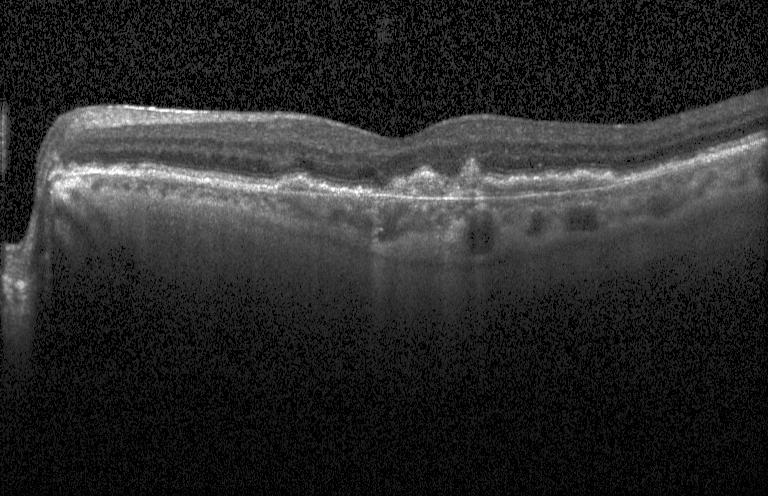 OCT B-scan. Impression: choroidal neovascularization (CNV).